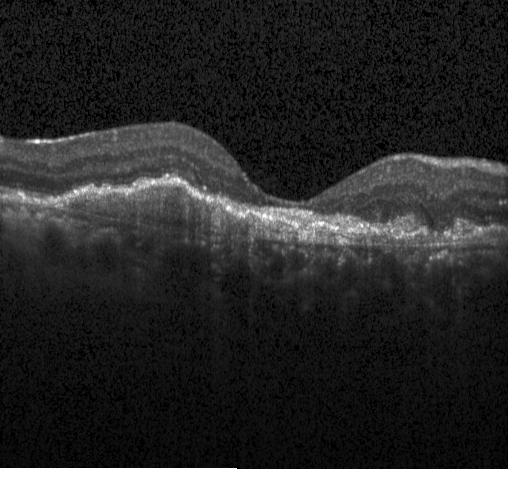 Retinal OCT B-scan — Finding: a choroidal neovascular membrane.